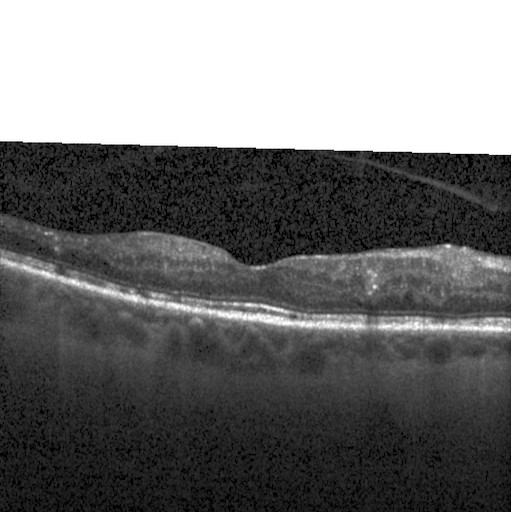

Dx: diabetic macular edema.